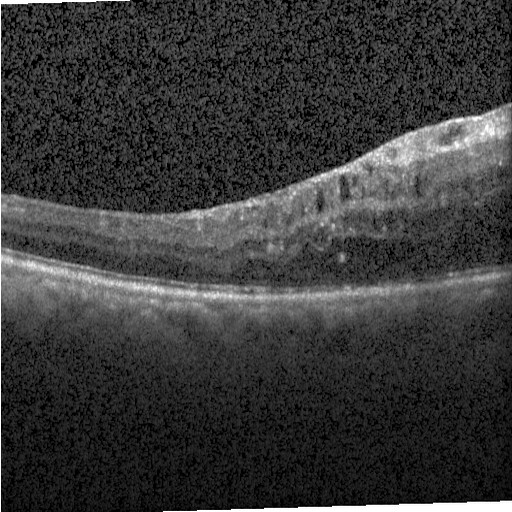

Centered on the fovea; OCT B-scan; spectral-domain optical coherence tomography. The scan shows diabetic macular edema.